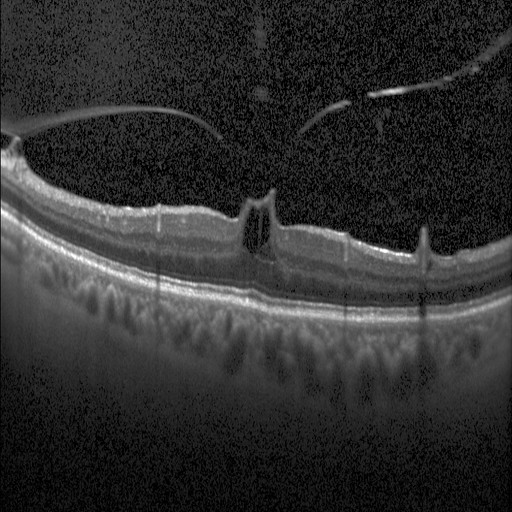

Impression: DME.